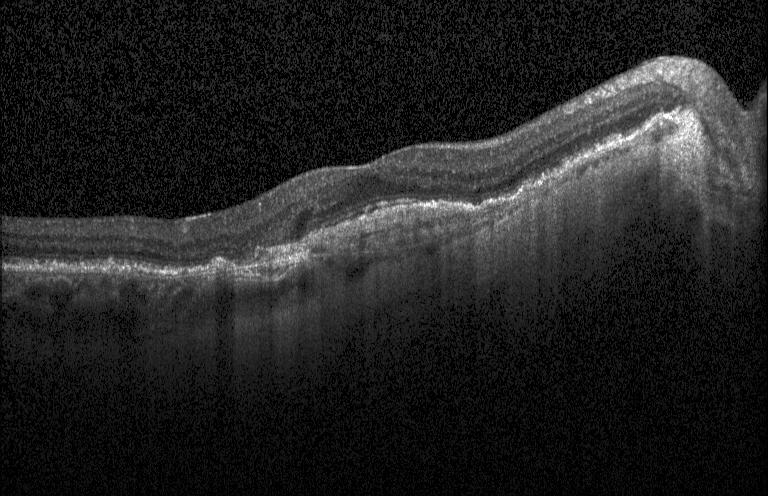

Macular OCT: choroidal neovascularization.